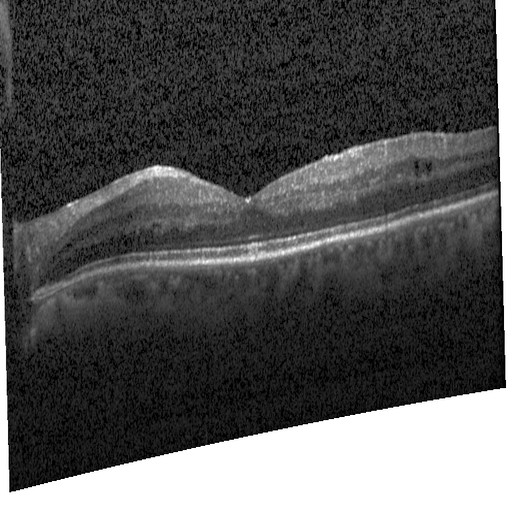 Diabetic macular edema.